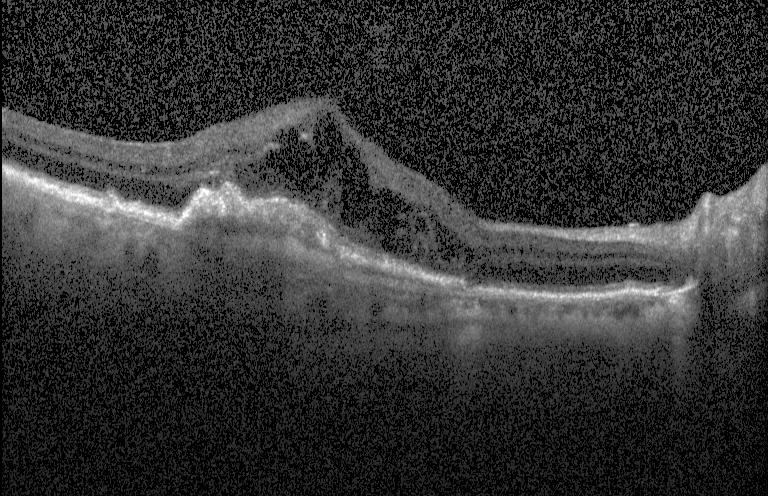 Finding: CNV.